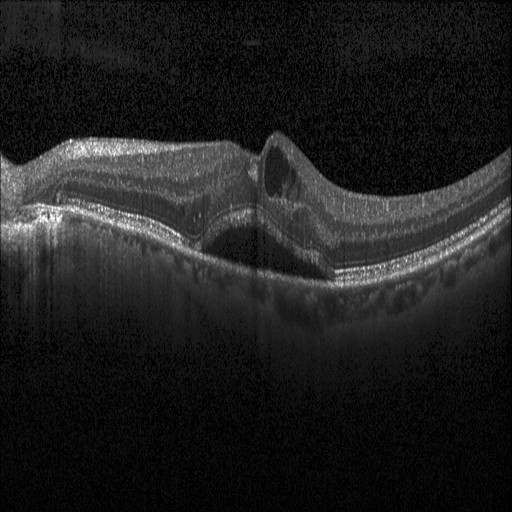
Impression: diabetic macular edema (DME).